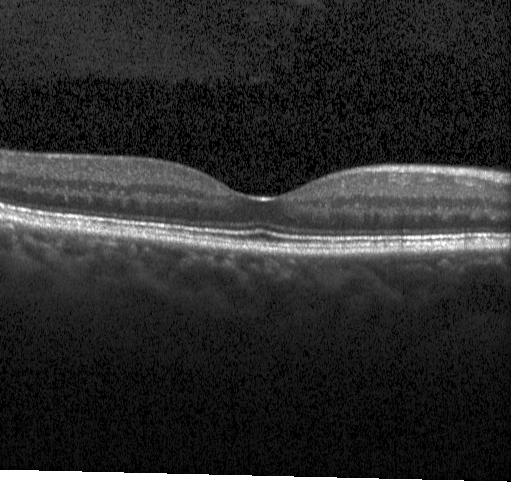
Horizontal scan through the fovea. Optical coherence tomography B-scan — No choroidal neovascularization, diabetic macular edema, or drusen.